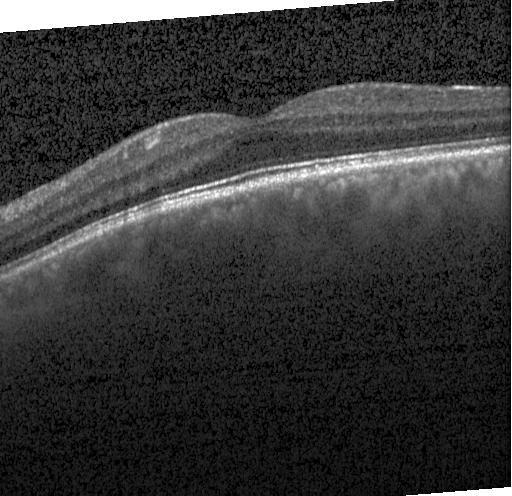 Retinal OCT B-scan. Macular scan. Spectral-domain optical coherence tomography. Heidelberg Spectralis OCT system. Diagnosis: no CNV, no DME, and no drusen.